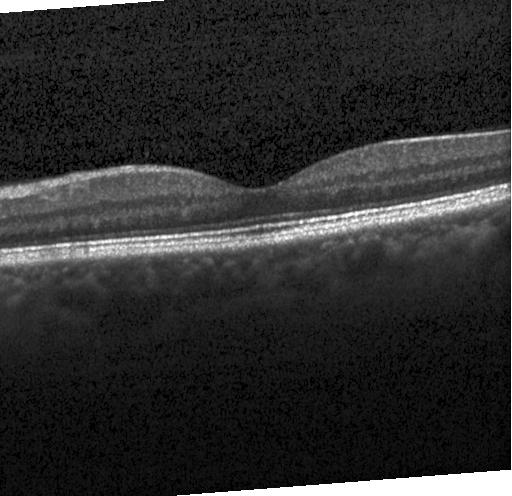
Finding: neither choroidal neovascularization, diabetic macular edema, nor drusen.